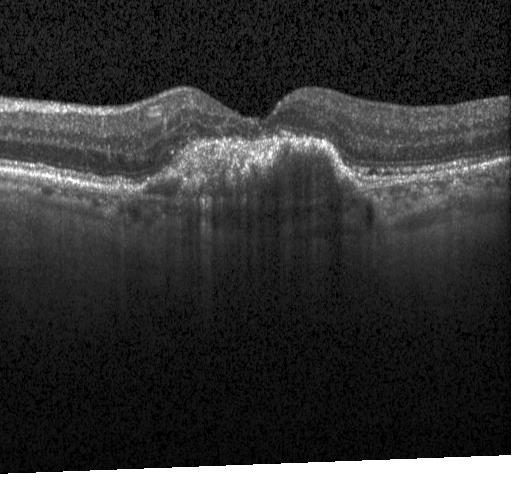 Diagnosis: choroidal neovascularization.